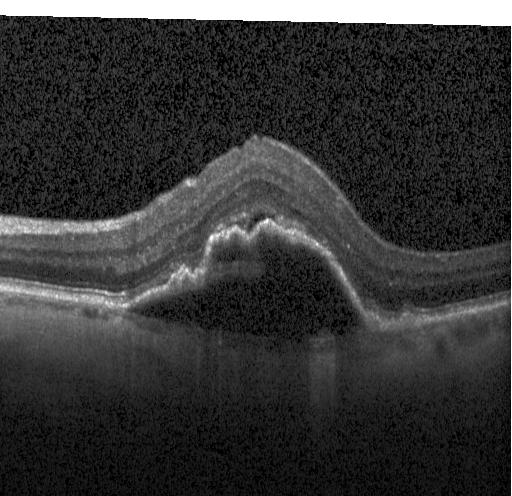
Optical coherence tomography scan — CNV.